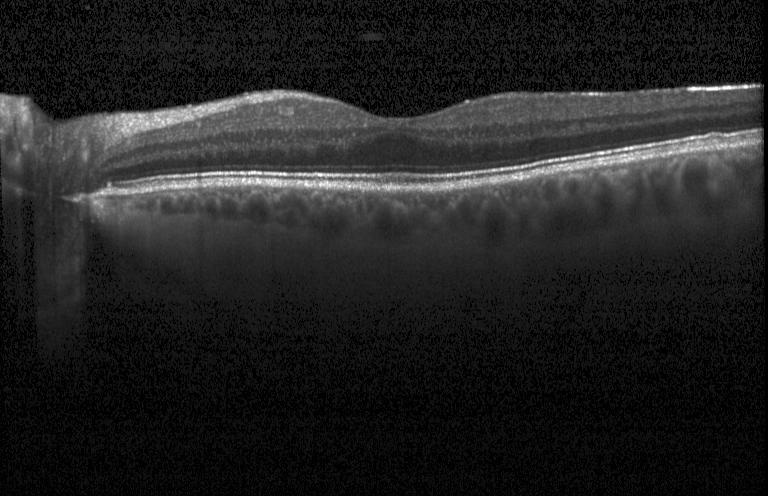
Dx: no choroidal neovascularization, diabetic macular edema, or drusen.